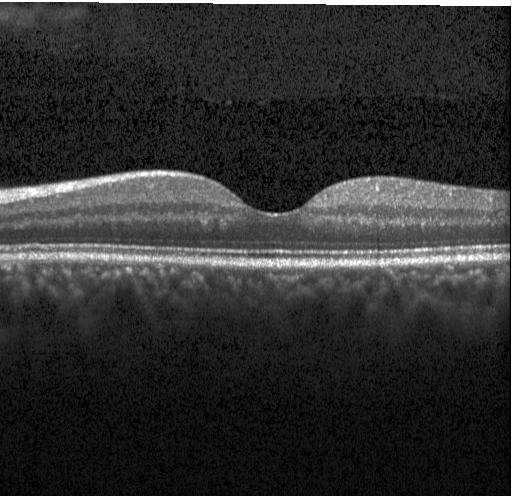 Optical coherence tomography scan.
No choroidal neovascularization, diabetic macular edema, or drusen.